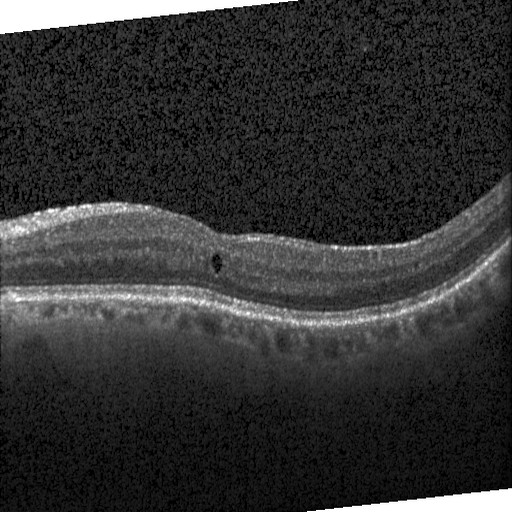

Impression: DME.